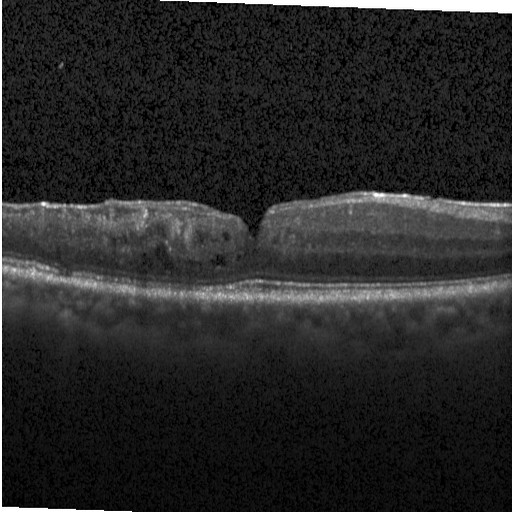 Spectral-domain optical coherence tomography. Optical coherence tomography B-scan. Through the macula. This B-scan demonstrates diabetic macular edema (DME).